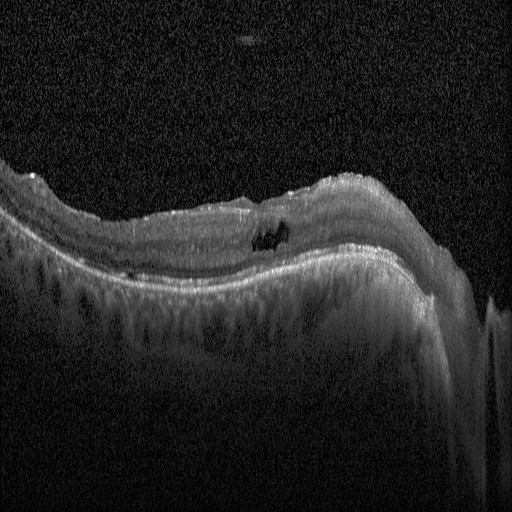

Dx: DME.